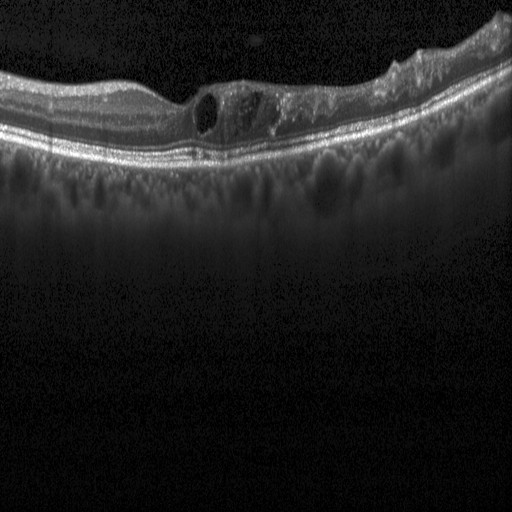
Optical coherence tomography B-scan.
The scan shows DME.